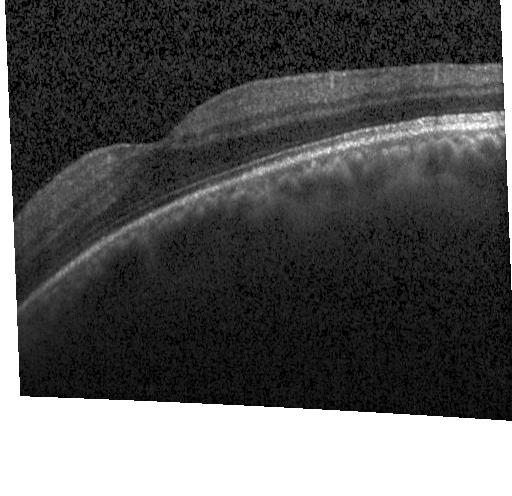

Assessment: no choroidal neovascularization, diabetic macular edema, or drusen.